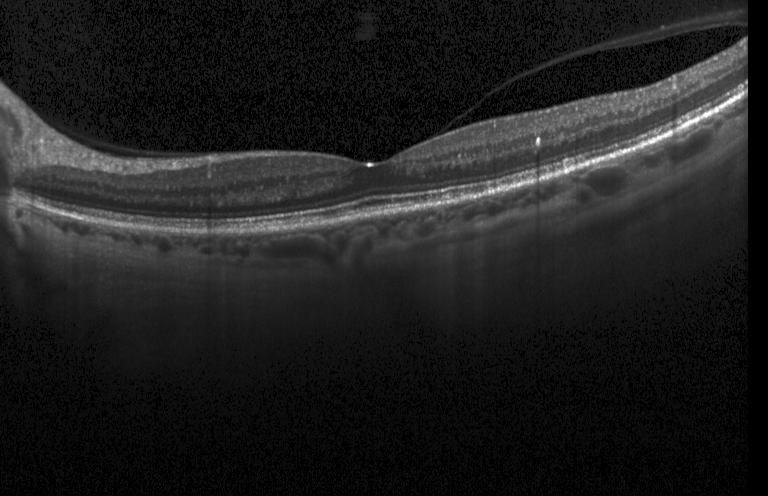

No choroidal neovascularization, no diabetic macular edema, and no drusen.